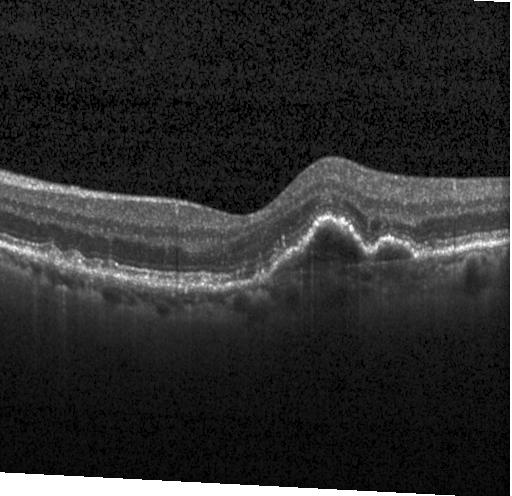

Finding: a choroidal neovascular membrane.